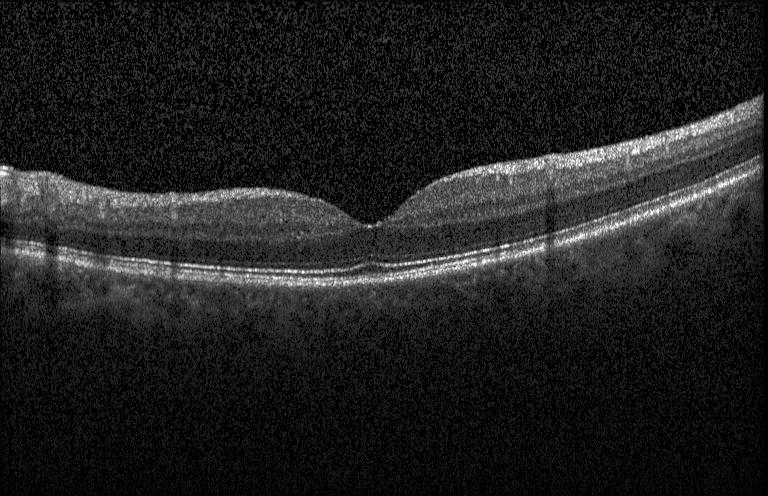 OCT finding: neither choroidal neovascularization, diabetic macular edema, nor drusen.